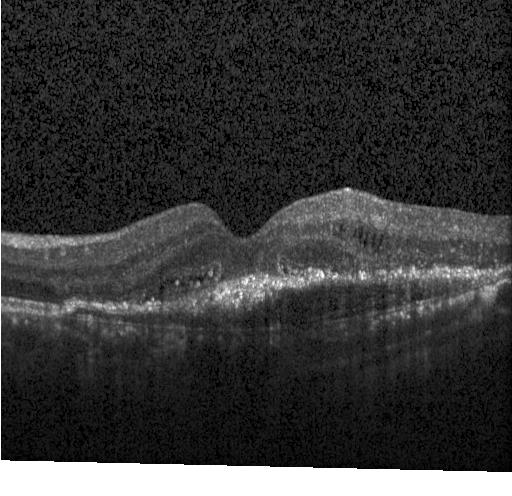
OCT scan showing a choroidal neovascular membrane.